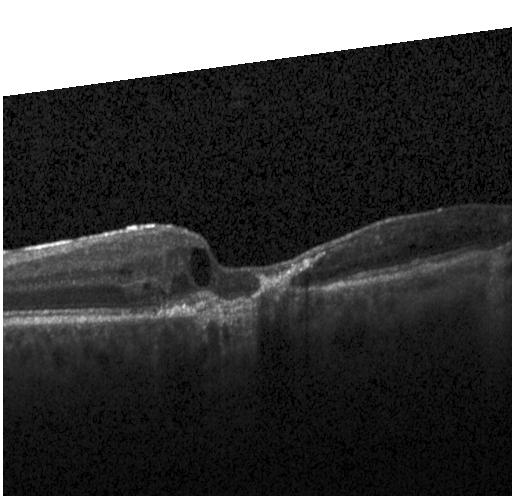

Centered on the fovea; acquired on a Heidelberg Spectralis; spectral-domain OCT; OCT B-scan.
Dx: choroidal neovascularization.